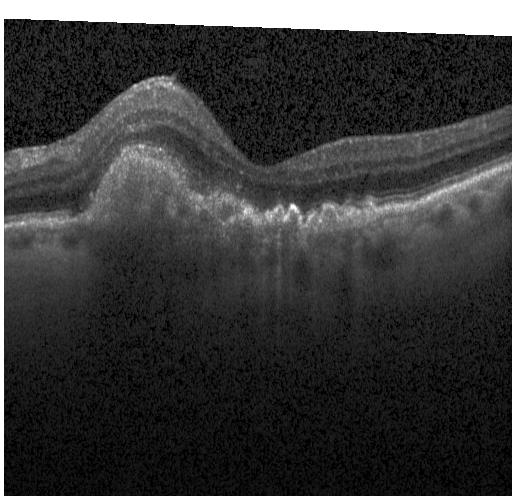
Spectral-domain OCT; retinal OCT cross-section; Heidelberg Spectralis OCT system; macular scan — Assessment: a choroidal neovascular membrane.